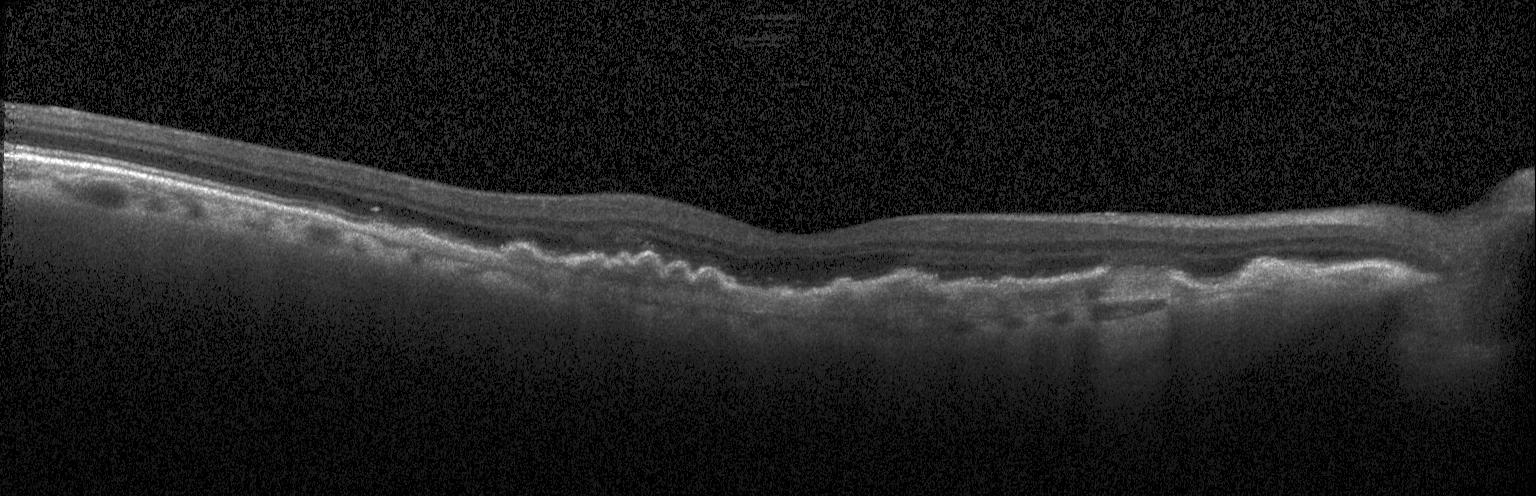
SD-OCT, through the macula, instrument: Heidelberg Spectralis, optical coherence tomography scan.
Diagnosis: choroidal neovascularization (CNV).